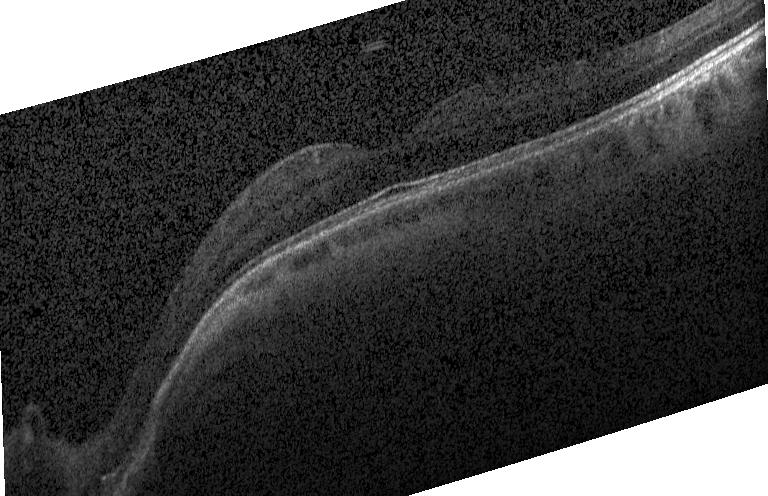

SD-OCT; OCT B-scan.
No evidence of choroidal neovascularization, diabetic macular edema, or drusen.